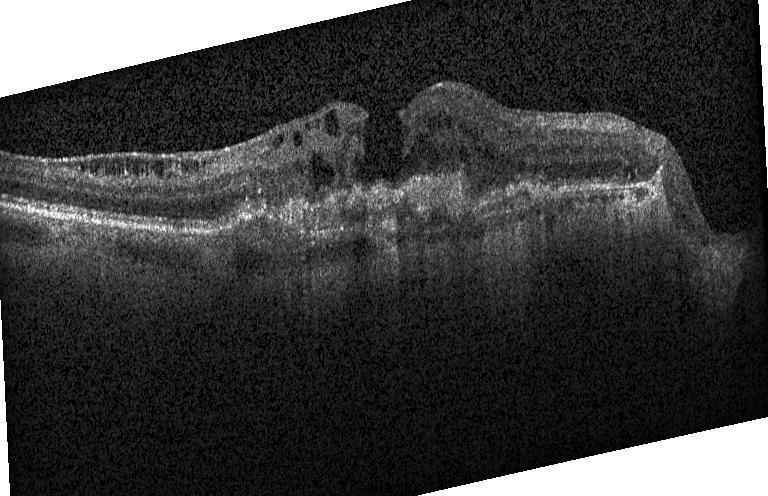 OCT B-scan. Assessment: a choroidal neovascular membrane.